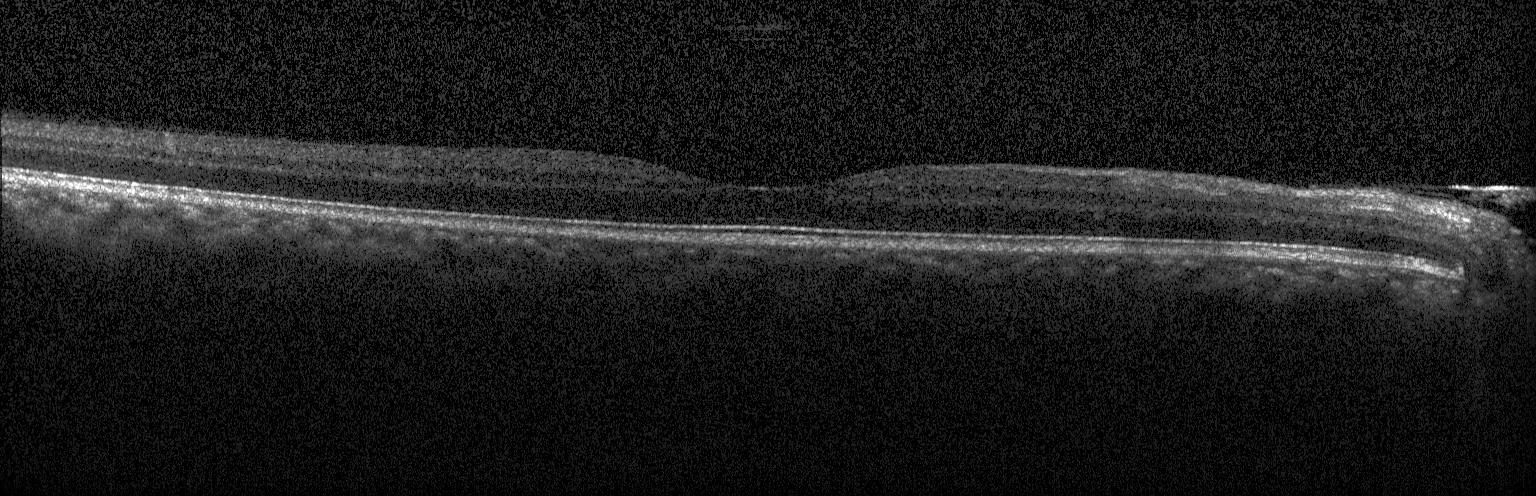
Macular scan. Heidelberg Spectralis OCT system. SD-OCT. OCT line scan — Macular OCT: no choroidal neovascularization, diabetic macular edema, or drusen.